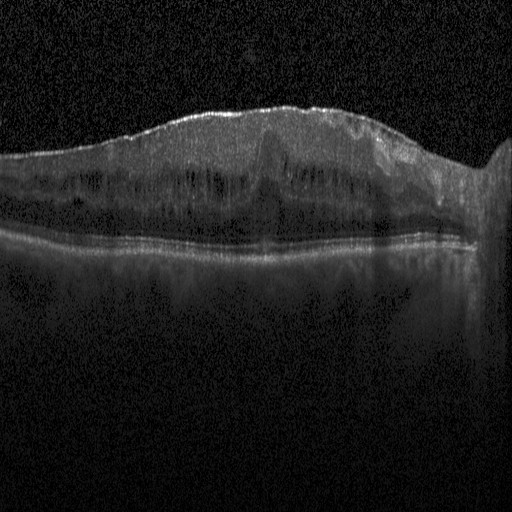

SD-OCT. Retinal OCT cross-section. Acquired on a Heidelberg Spectralis. Diabetic macular edema (DME).